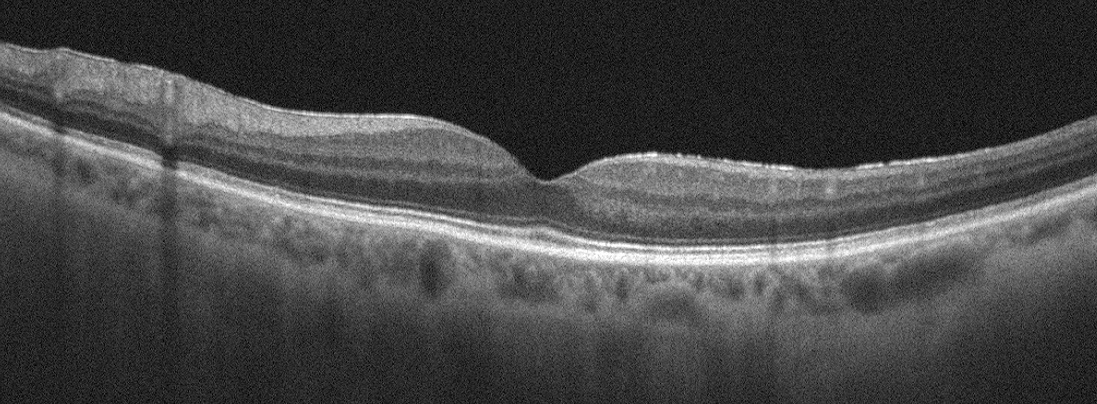 This B-scan demonstrates epiretinal membrane (ERM).